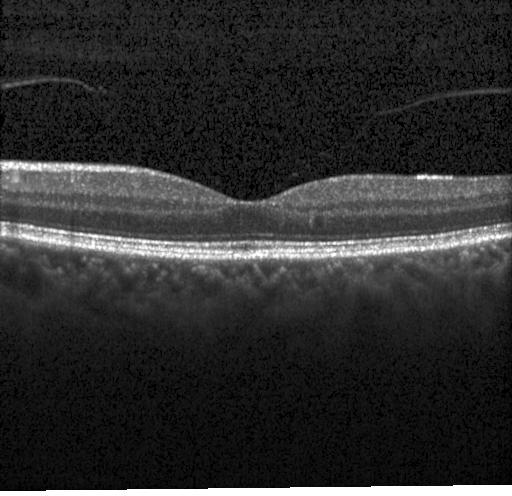
Heidelberg Spectralis OCT system · centered on the fovea · SD-OCT · optical coherence tomography scan. No evidence of CNV, DME, or drusen.